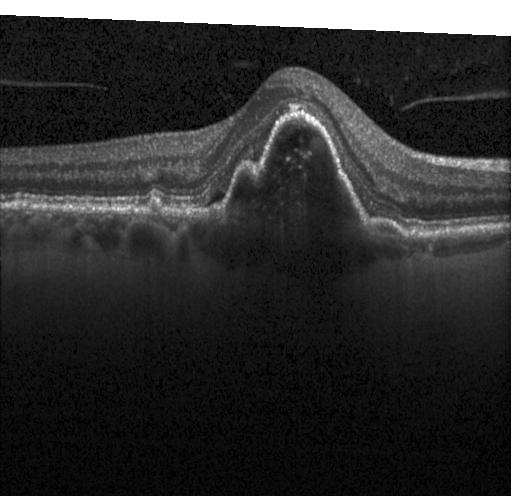
Retinal OCT cross-section. Dx: a choroidal neovascular membrane.